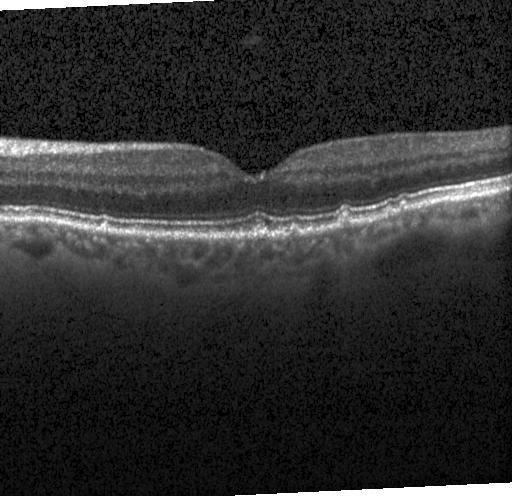

Macular scan. Spectral-domain OCT. Optical coherence tomography scan. Heidelberg Spectralis OCT system — This B-scan demonstrates multiple drusen.